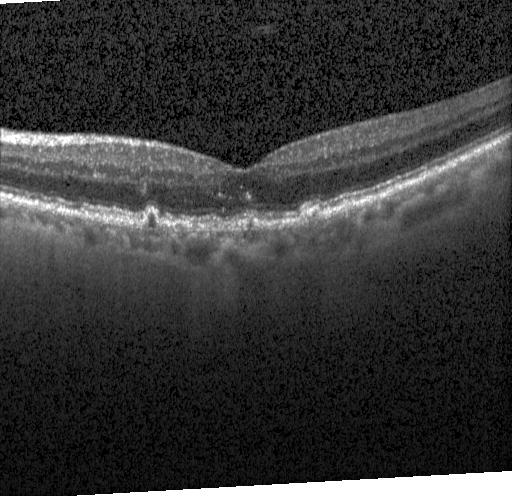 Optical coherence tomography scan, through the macula — Assessment: choroidal neovascularization.